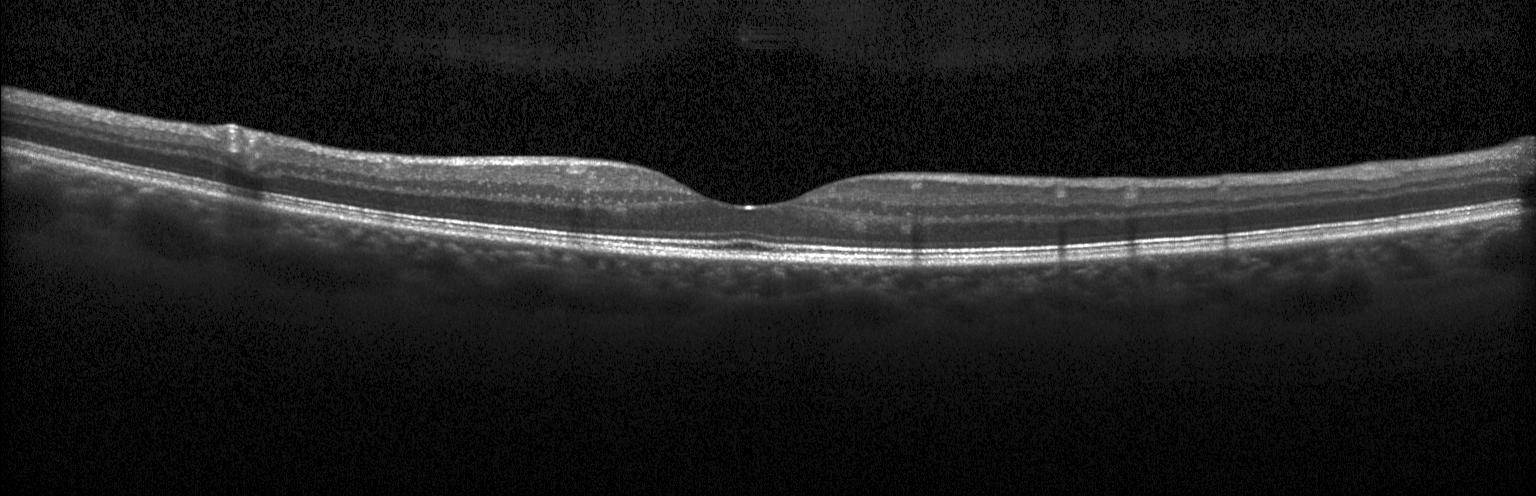

SD-OCT · fovea-centered · instrument: Heidelberg Spectralis · OCT B-scan — Diagnosis: no evidence of CNV, DME, or drusen.